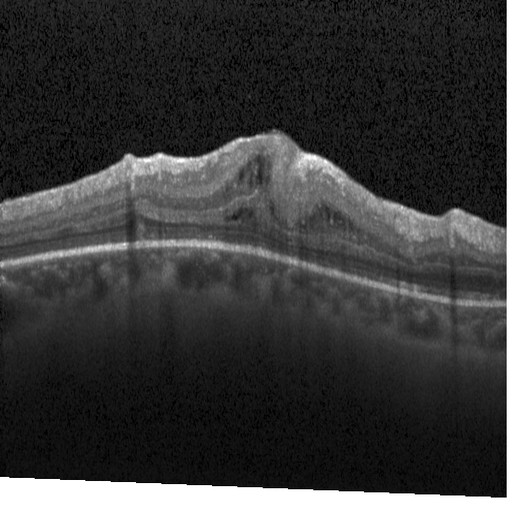
Macular OCT demonstrating diabetic macular edema (DME).